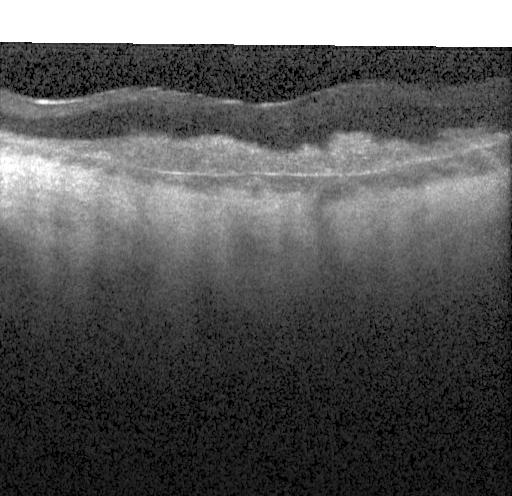

Heidelberg Spectralis, SD-OCT, OCT line scan
Impression: a choroidal neovascular membrane.